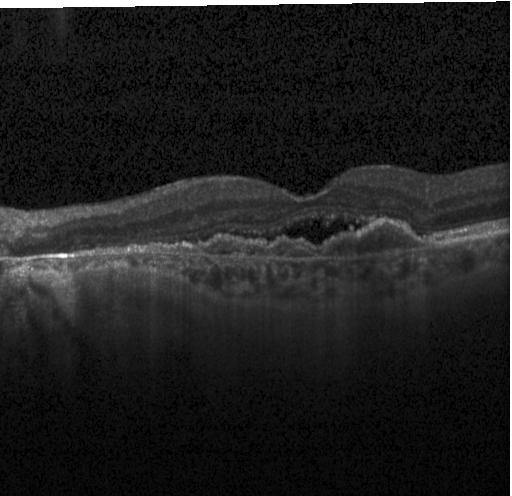 Macular scan. Acquired on a Heidelberg Spectralis. Retinal OCT cross-section.
Diagnosis: a choroidal neovascular membrane.